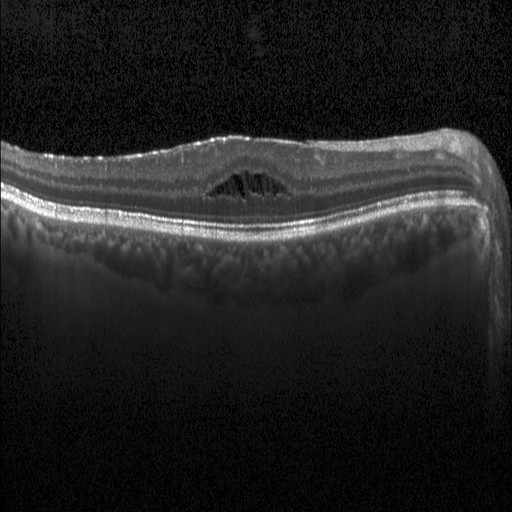

Instrument: Heidelberg Spectralis, optical coherence tomography B-scan, spectral-domain optical coherence tomography
Diagnosis: diabetic macular edema (DME).